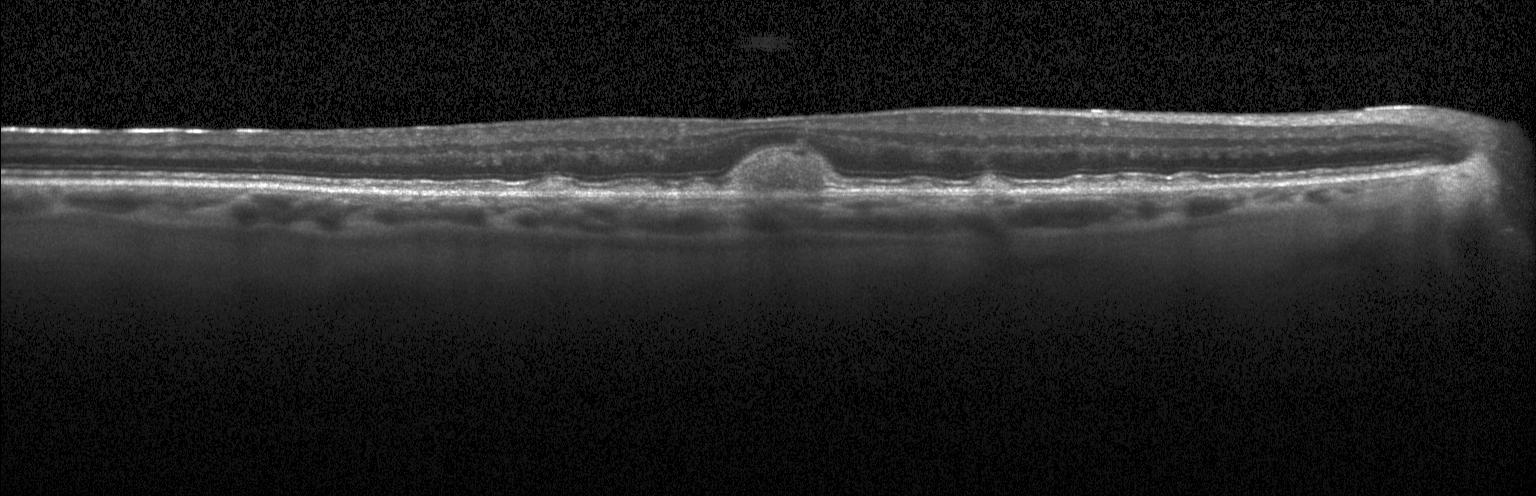

OCT scan showing a choroidal neovascular membrane.